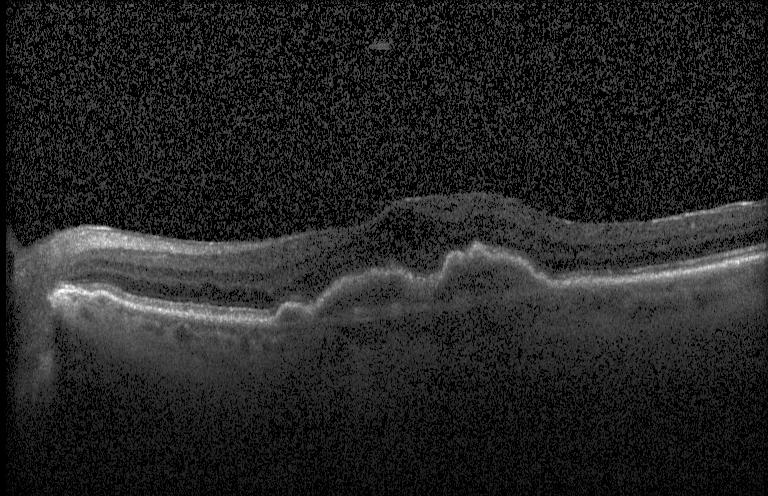 Impression: choroidal neovascularization (CNV).